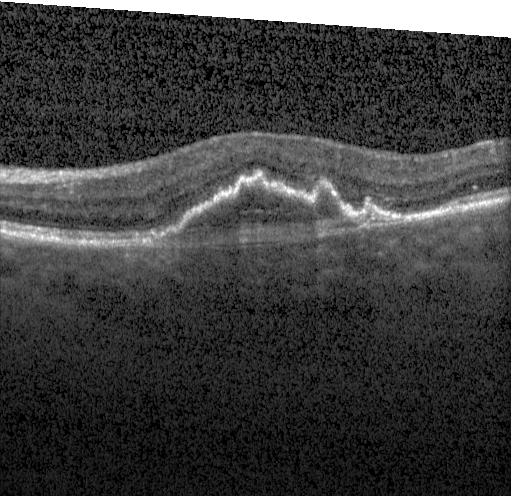 Optical coherence tomography scan — Assessment: choroidal neovascularization.